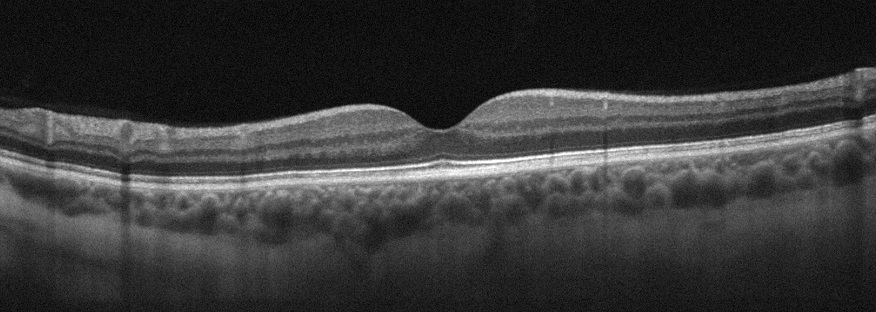
Diagnosis: absence of AMD, DME, ERM, RAO, RVO, and vitreomacular interface disease.